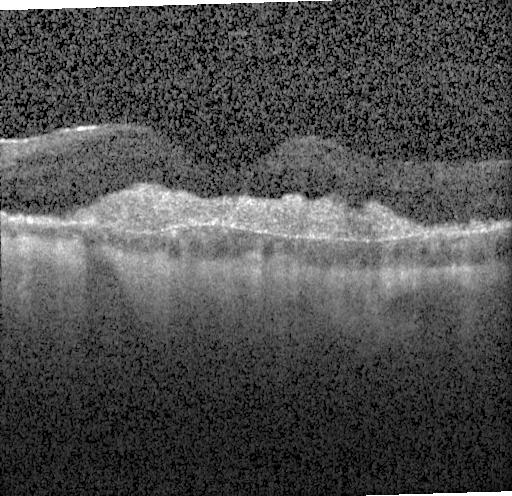

OCT B-scan.
Assessment: choroidal neovascularization.